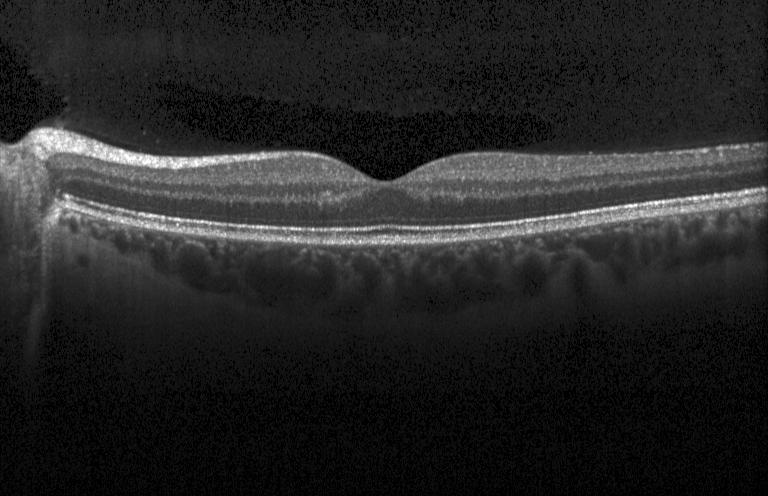 Neither CNV, DME, nor drusen.